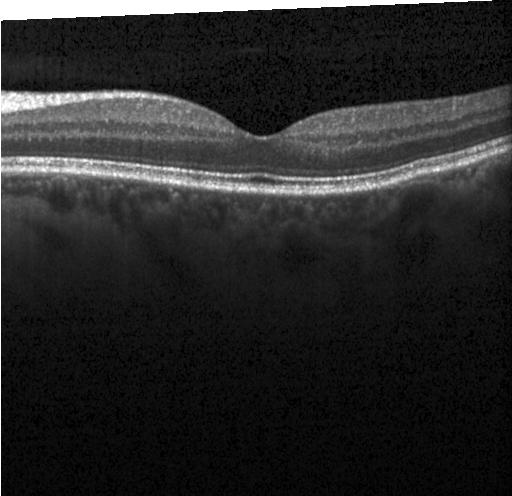

Optical coherence tomography B-scan.
This B-scan demonstrates no choroidal neovascularization, diabetic macular edema, or drusen.